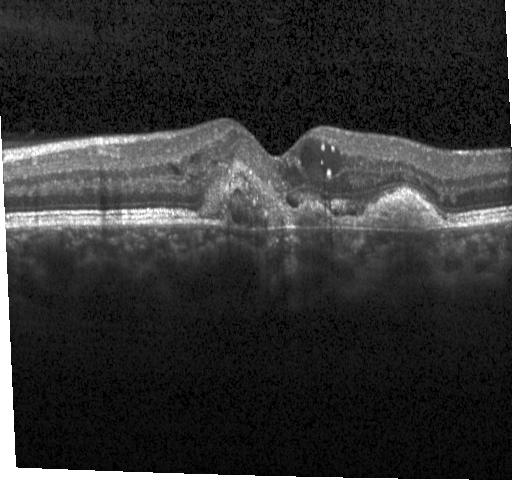
Macular scan. Spectral-domain optical coherence tomography. OCT line scan. Instrument: Heidelberg Spectralis.
This B-scan demonstrates a choroidal neovascular membrane.